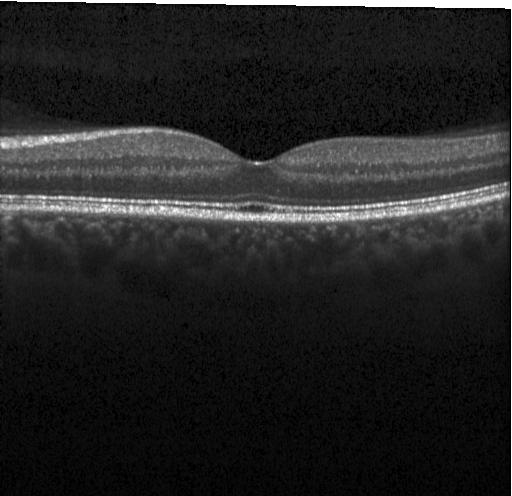

Spectral-domain OCT · optical coherence tomography B-scan · horizontal scan through the fovea
This B-scan demonstrates no CNV, DME, or drusen.